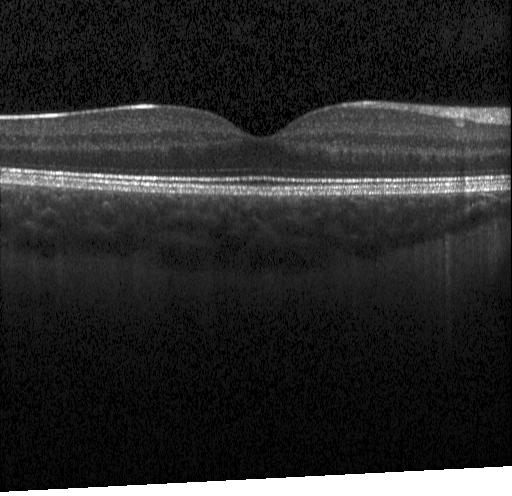

Diagnosis: no CNV, no DME, and no drusen.